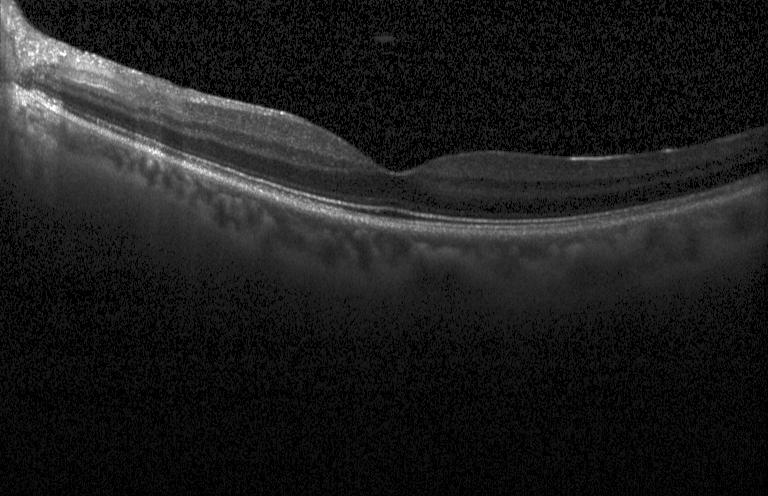
OCT B-scan
Diagnosis: no CNV, DME, or drusen.